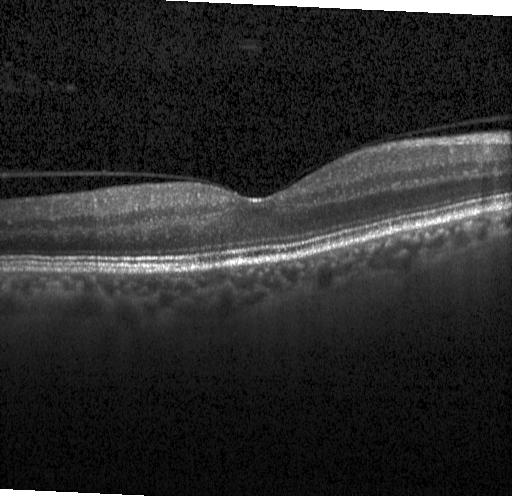 Retinal OCT cross-section. Assessment: no evidence of choroidal neovascularization, diabetic macular edema, or drusen.